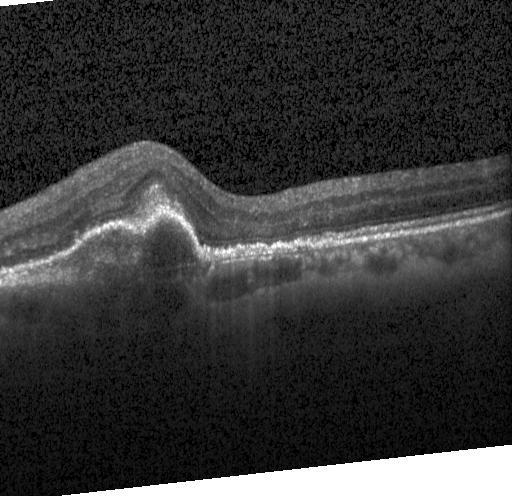 Assessment: a choroidal neovascular membrane.